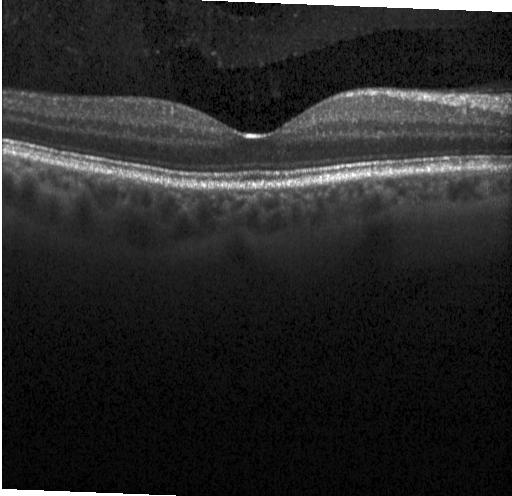
Optical coherence tomography B-scan · macular scan · Heidelberg Spectralis.
OCT finding: neither choroidal neovascularization, diabetic macular edema, nor drusen.